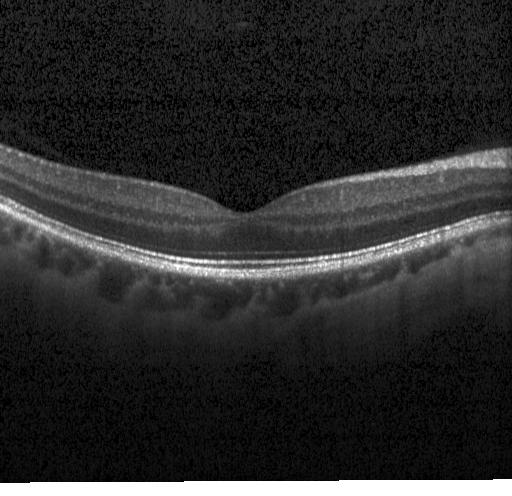

OCT B-scan, spectral-domain OCT, Heidelberg Spectralis
Finding: no choroidal neovascularization, diabetic macular edema, or drusen.